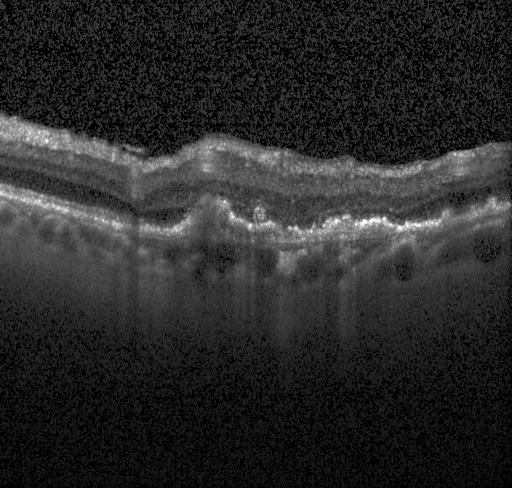
Retinal OCT B-scan · centered on the fovea.
OCT finding: a choroidal neovascular membrane.